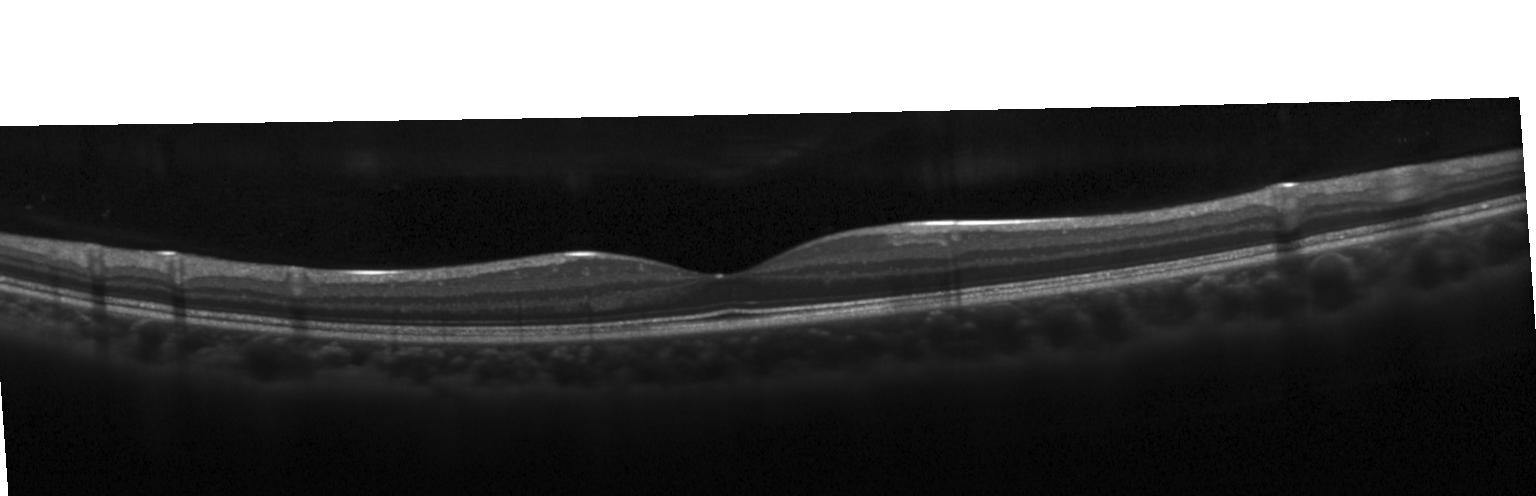 The scan shows neither choroidal neovascularization, diabetic macular edema, nor drusen.